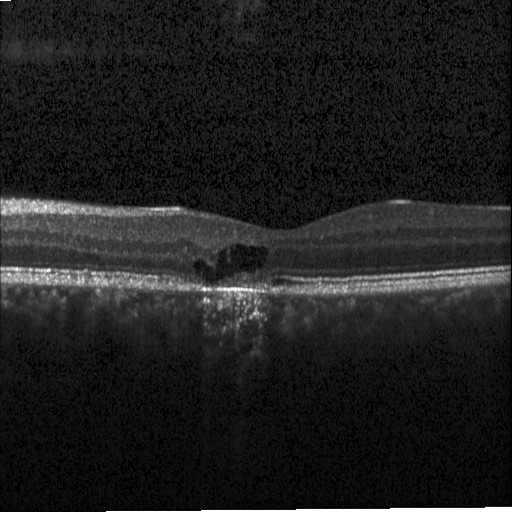

Dx: diabetic macular edema.